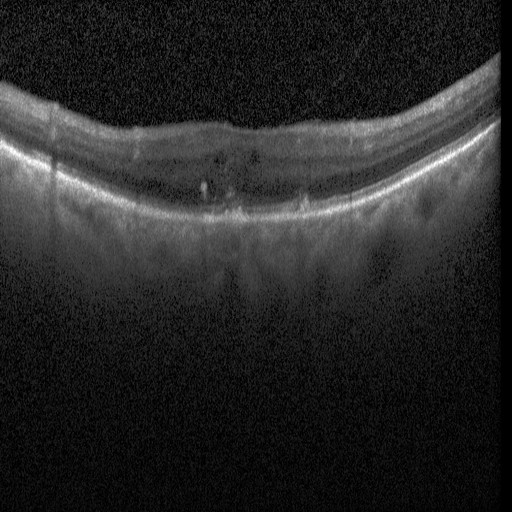 OCT scan showing diabetic macular edema (DME).